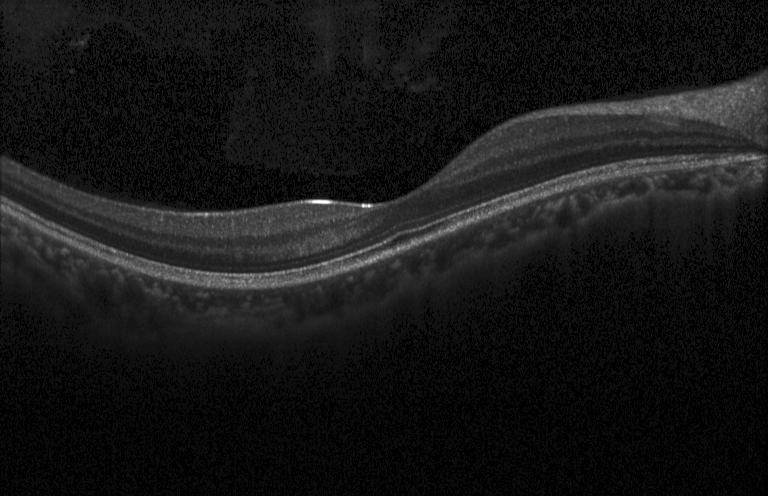
Dx: neither choroidal neovascularization, diabetic macular edema, nor drusen.